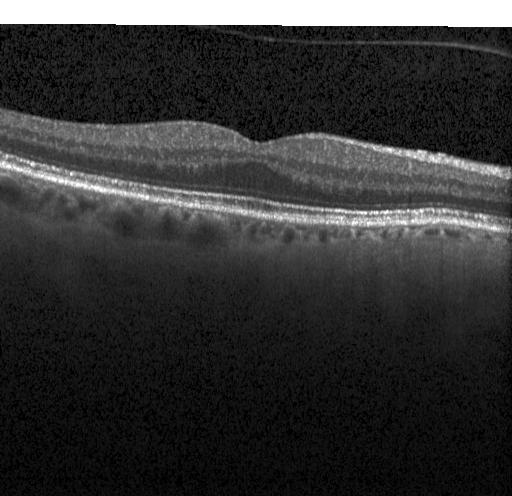
Retinal OCT B-scan · instrument: Heidelberg Spectralis · horizontal scan through the fovea.
This B-scan demonstrates no CNV, no DME, and no drusen.